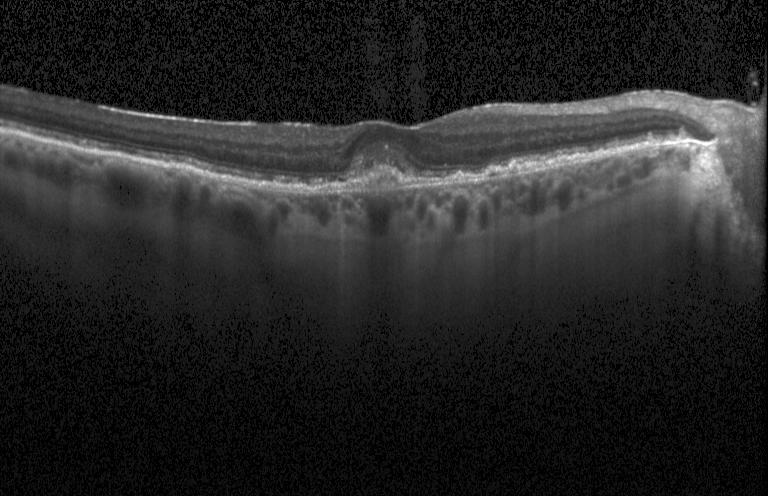
Instrument: Heidelberg Spectralis, OCT B-scan, macular scan, spectral-domain OCT.
A choroidal neovascular membrane.